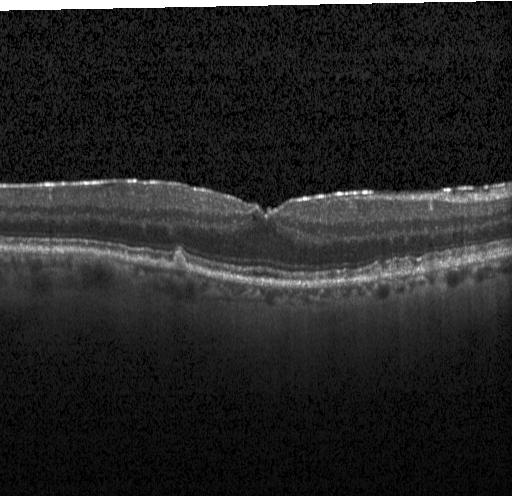 OCT line scan.
Diagnosis: drusen.